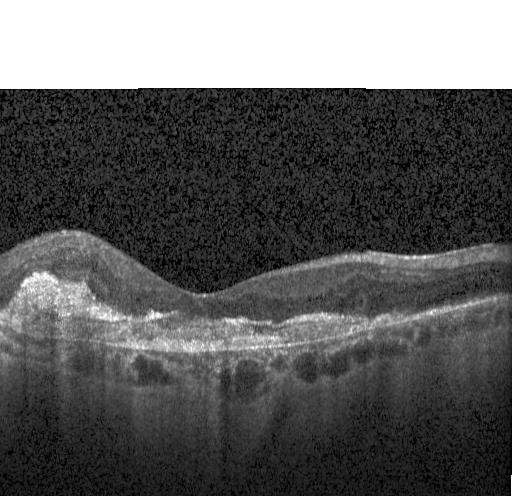

Optical coherence tomography scan.
Diagnosis: choroidal neovascularization.